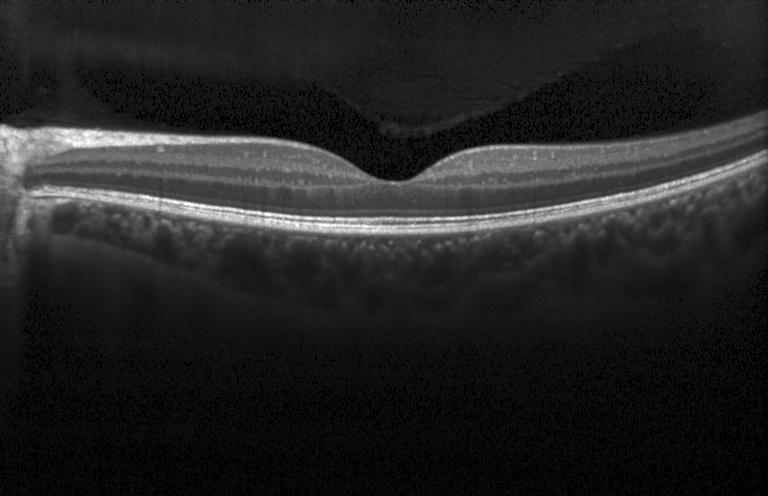

The scan shows no choroidal neovascularization, no diabetic macular edema, and no drusen.